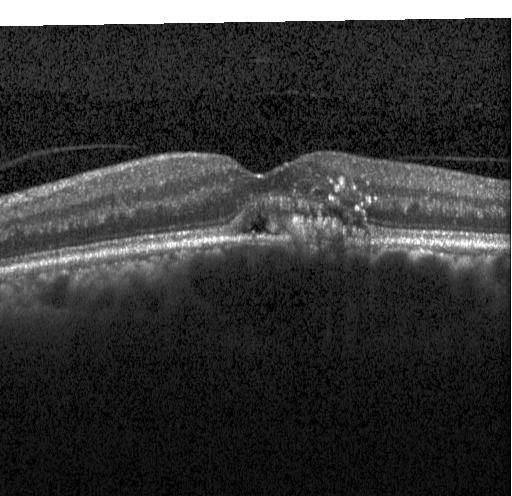
Retinal OCT B-scan — Diagnosis: choroidal neovascularization.